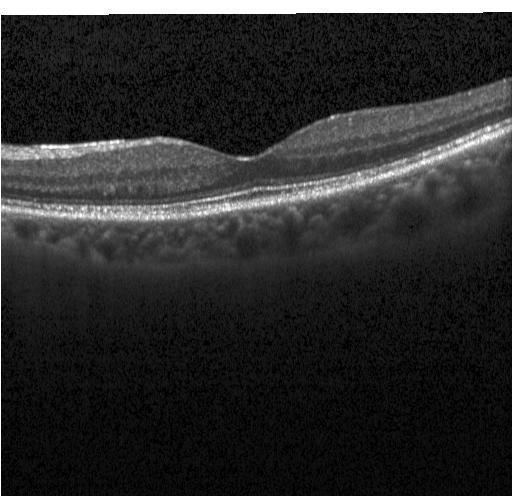

Macular OCT: no CNV, DME, or drusen.